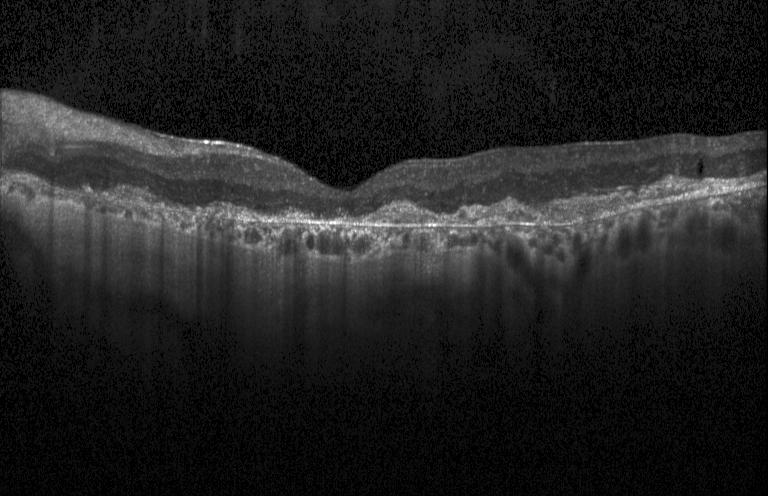

Retinal OCT cross-section; horizontal scan through the fovea.
Finding: CNV.